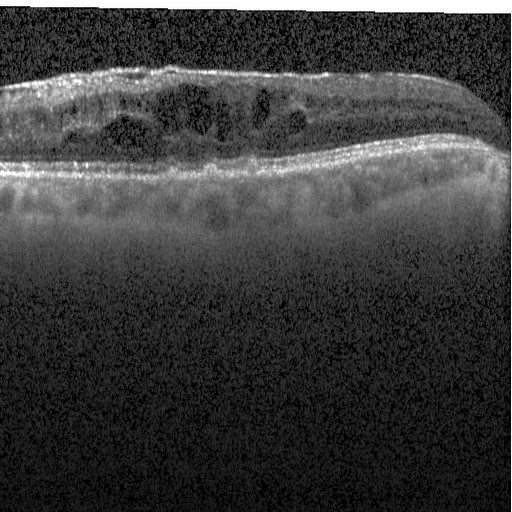 Macular OCT demonstrating diabetic macular edema (DME).